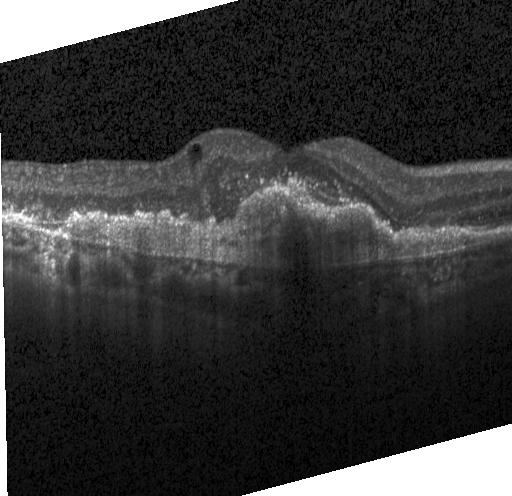 Diagnosis: choroidal neovascularization (CNV).